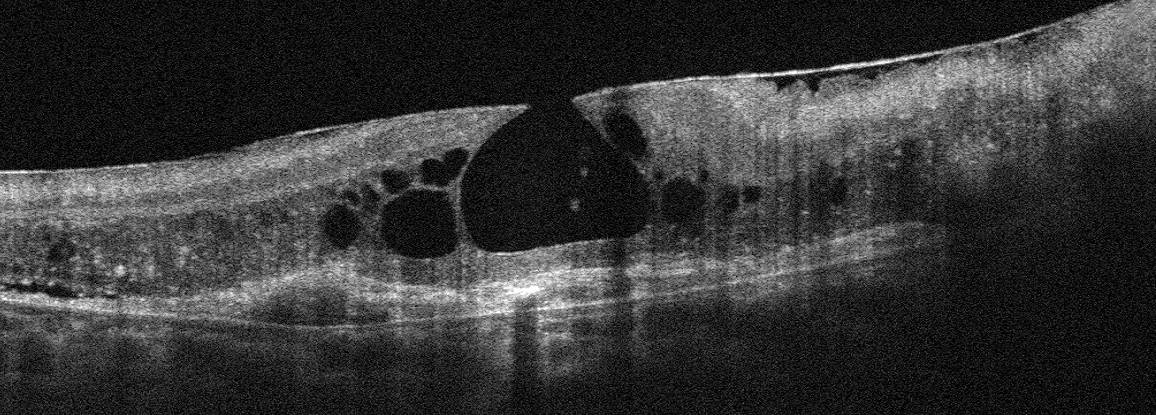
Optical coherence tomography B-scan; macular scan; Optovue Avanti RTVue XR
Impression: AMD.